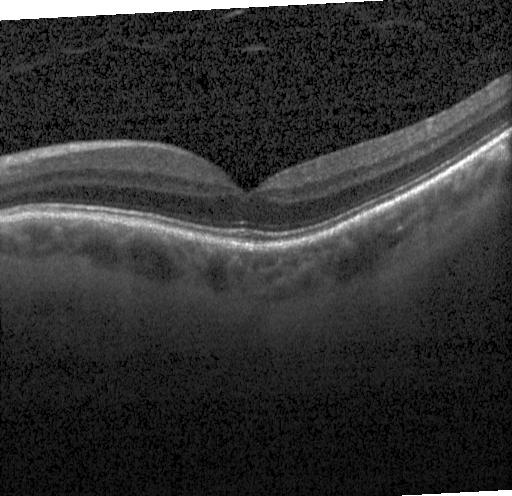
OCT line scan — Finding: no evidence of choroidal neovascularization, diabetic macular edema, or drusen.